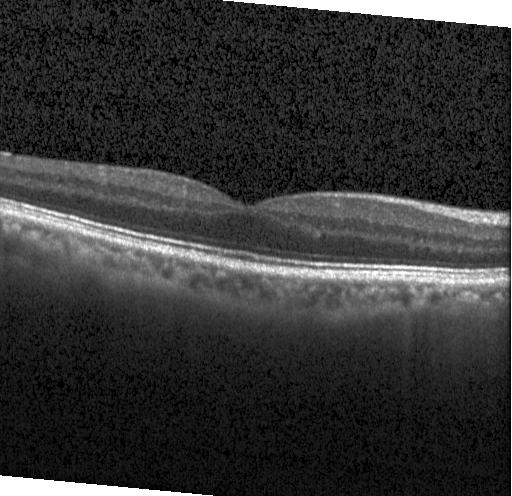
Impression: neither choroidal neovascularization, diabetic macular edema, nor drusen.